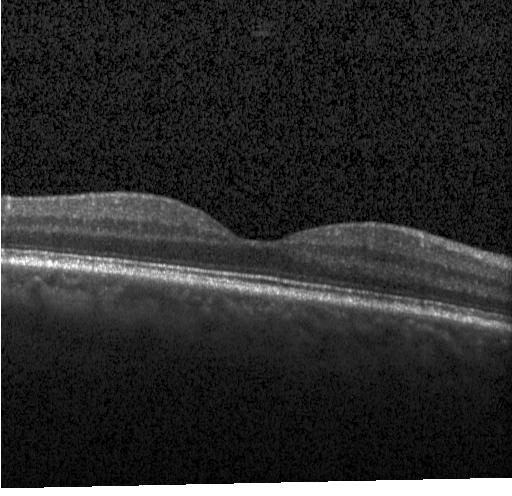

Diagnosis: no choroidal neovascularization, no diabetic macular edema, and no drusen.